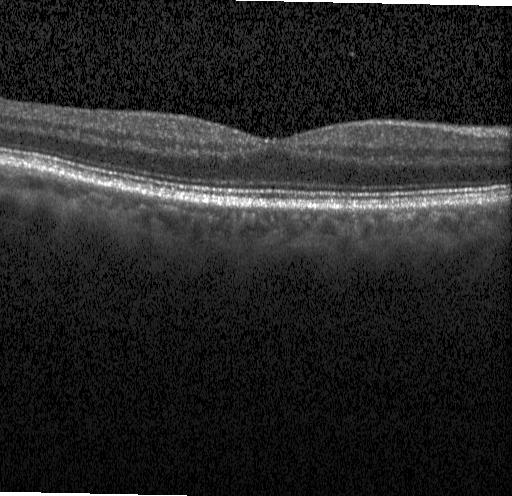

Retinal OCT cross-section — Impression: no choroidal neovascularization, diabetic macular edema, or drusen.